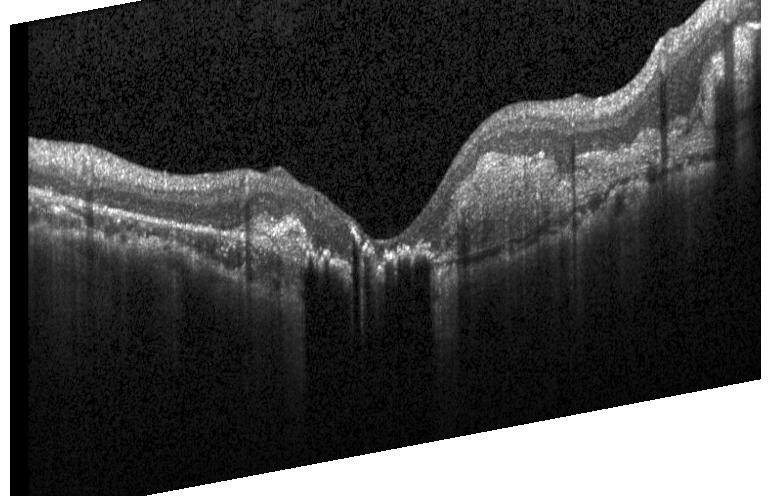

Spectral-domain OCT B-scan: choroidal neovascularization.